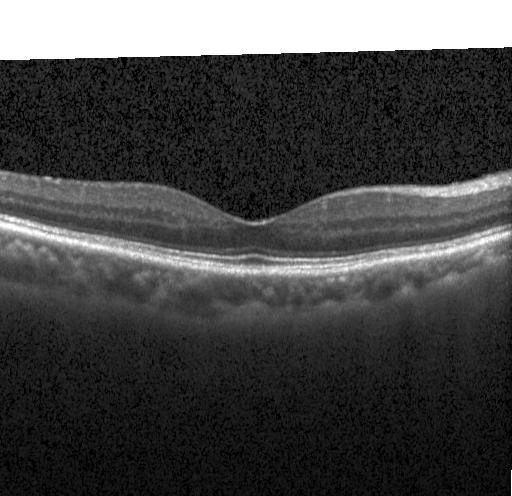

Macular OCT: no CNV, DME, or drusen.